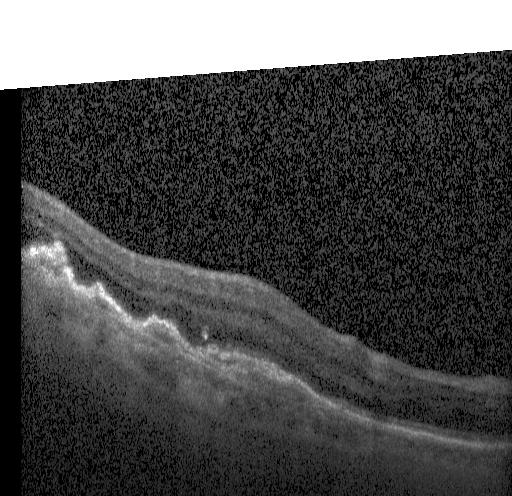
Instrument: Heidelberg Spectralis. OCT line scan. Horizontal scan through the fovea. Spectral-domain OCT. Diagnosis: a choroidal neovascular membrane.